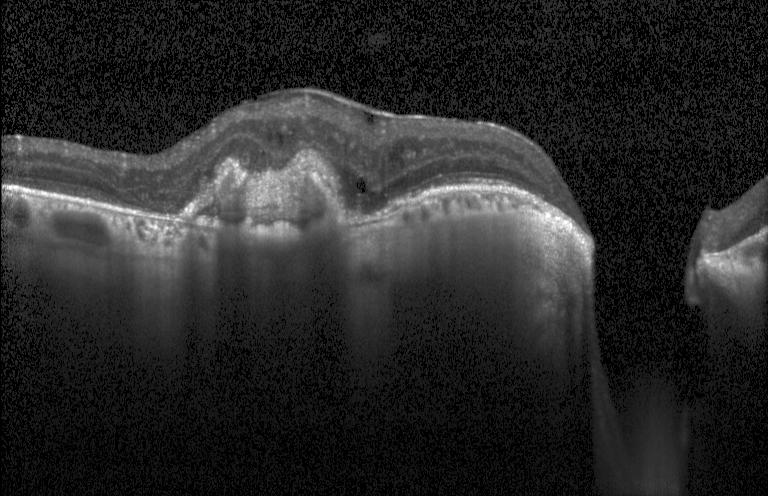 Impression: CNV.